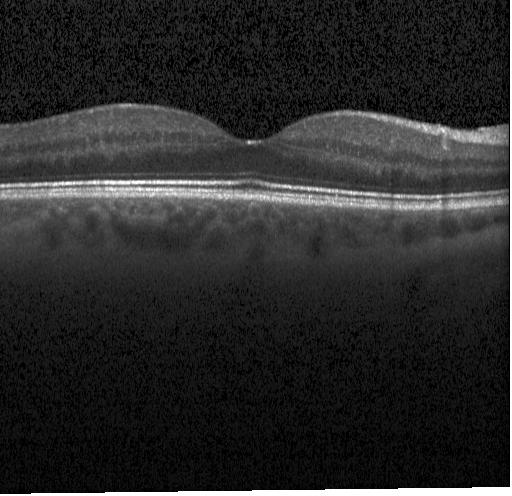
Impression: no CNV, DME, or drusen.